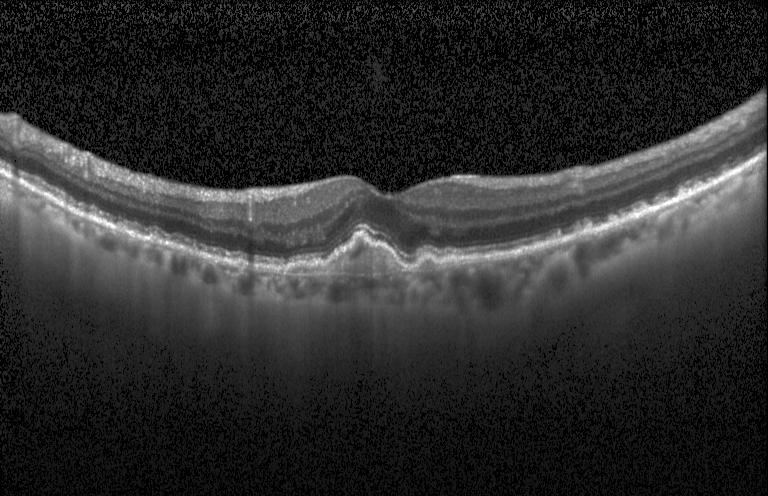

Optical coherence tomography scan; macular scan — Assessment: CNV.